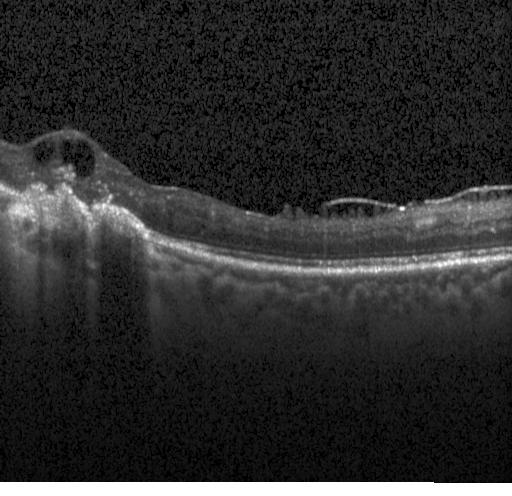 Retinal OCT B-scan. CNV.